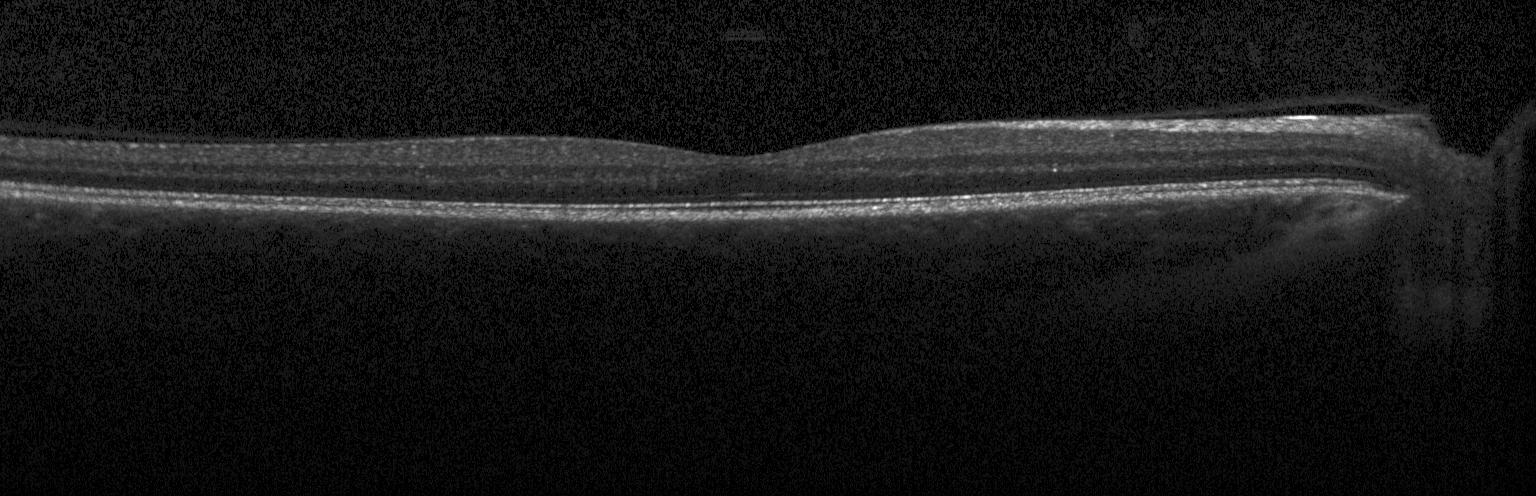

OCT B-scan; spectral-domain OCT; instrument: Heidelberg Spectralis — Diagnosis: no choroidal neovascularization, no diabetic macular edema, and no drusen.